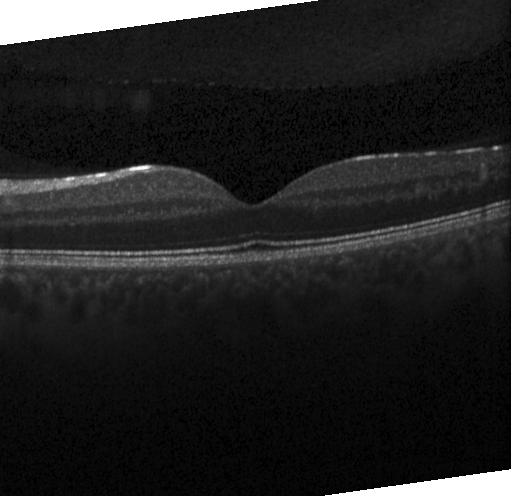
Instrument: Heidelberg Spectralis; SD-OCT; optical coherence tomography scan — Finding: no choroidal neovascularization, diabetic macular edema, or drusen.